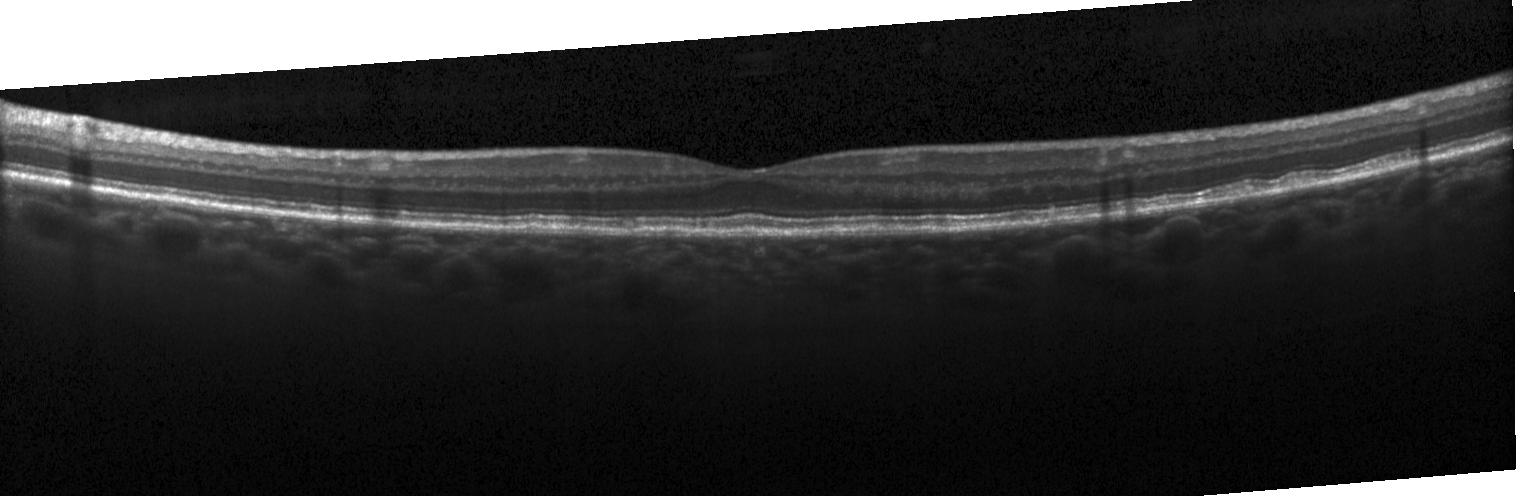 Heidelberg Spectralis OCT system · SD-OCT · OCT B-scan · fovea-centered
Impression: sub-RPE drusenoid deposits.